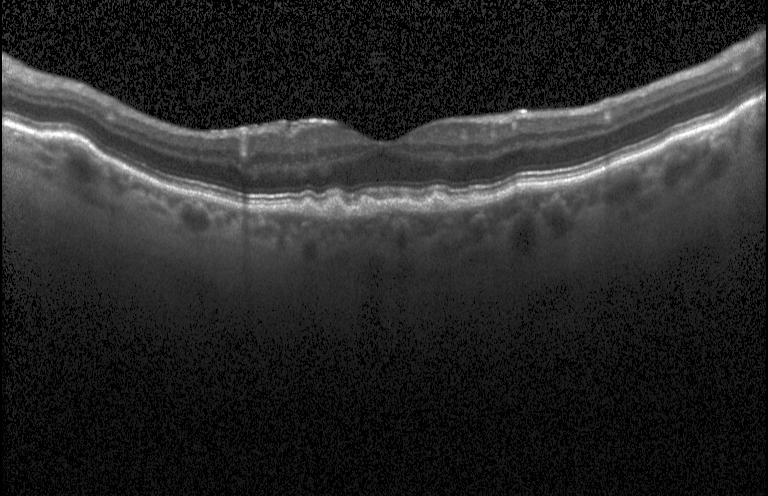

Instrument: Heidelberg Spectralis. OCT B-scan. Spectral-domain OCT. Horizontal scan through the fovea — Finding: multiple drusen.